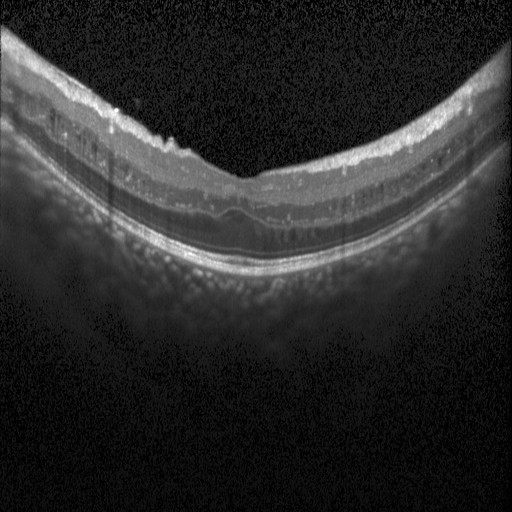 Retinal OCT cross-section.
Assessment: diabetic macular edema.